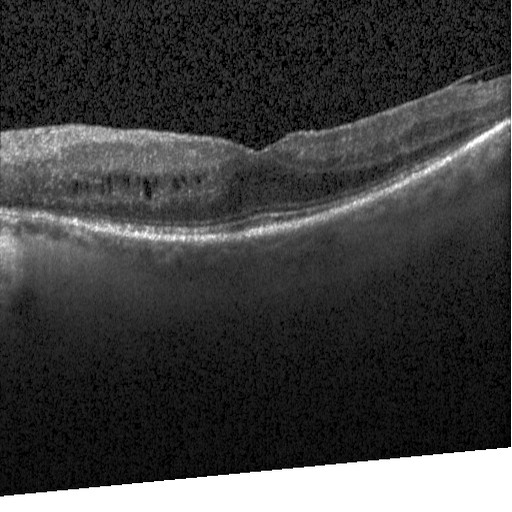

Retinal OCT cross-section, fovea-centered. This B-scan demonstrates diabetic macular edema (DME).